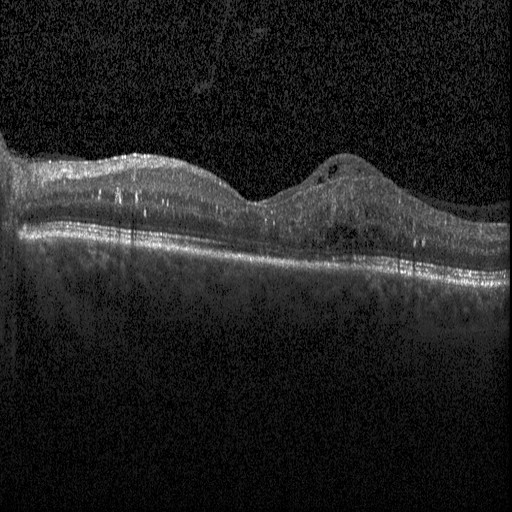
Retinal OCT B-scan — The scan shows diabetic macular edema.